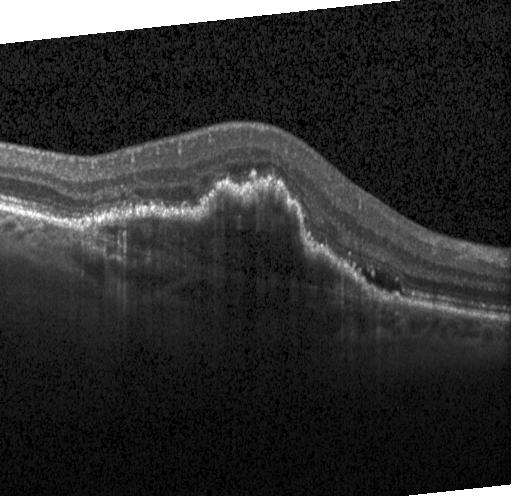

OCT B-scan showing a choroidal neovascular membrane.